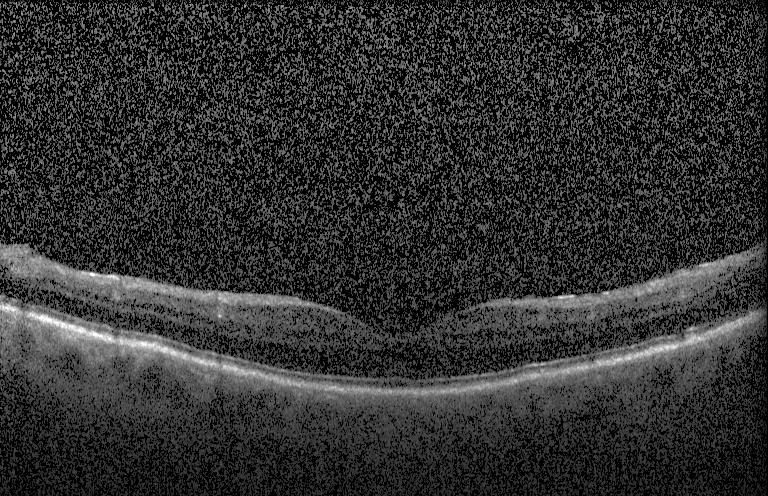

Impression: no evidence of choroidal neovascularization, diabetic macular edema, or drusen.